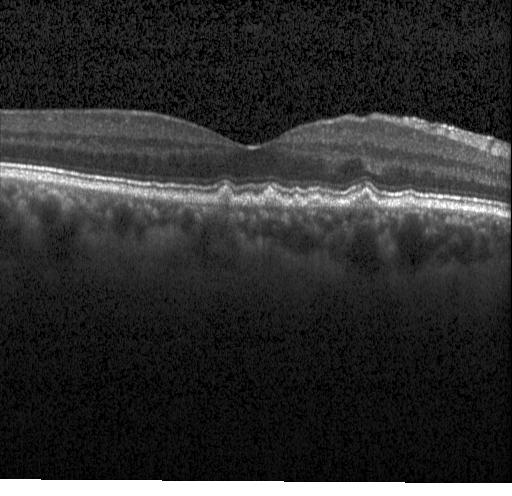
Heidelberg Spectralis. SD-OCT. OCT B-scan
Drusen.